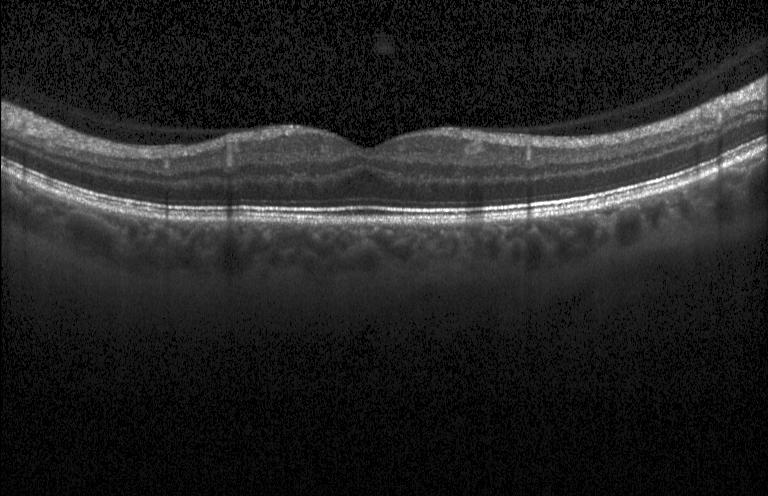
Finding: no choroidal neovascularization, diabetic macular edema, or drusen.